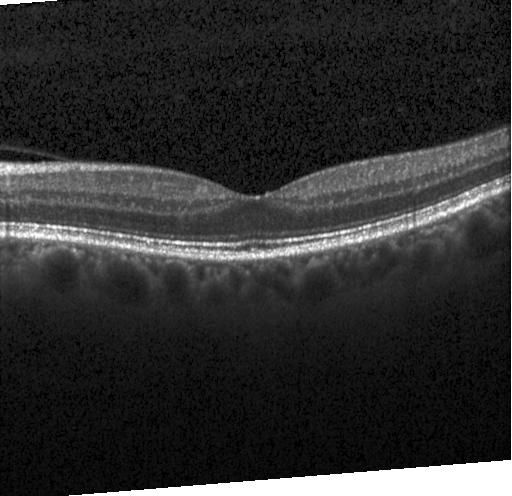 Dx: no evidence of choroidal neovascularization, diabetic macular edema, or drusen.